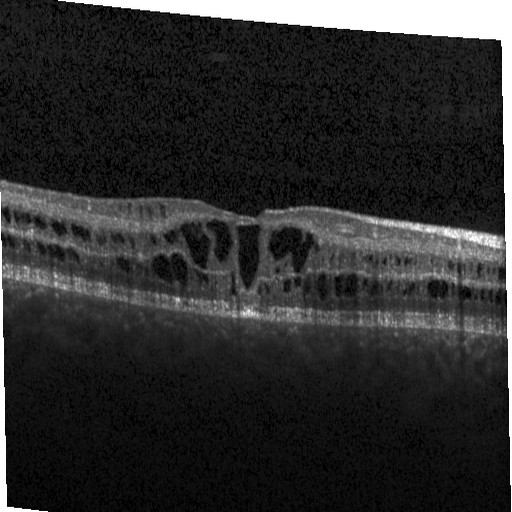
OCT line scan. Spectral-domain OCT — The scan shows DME.